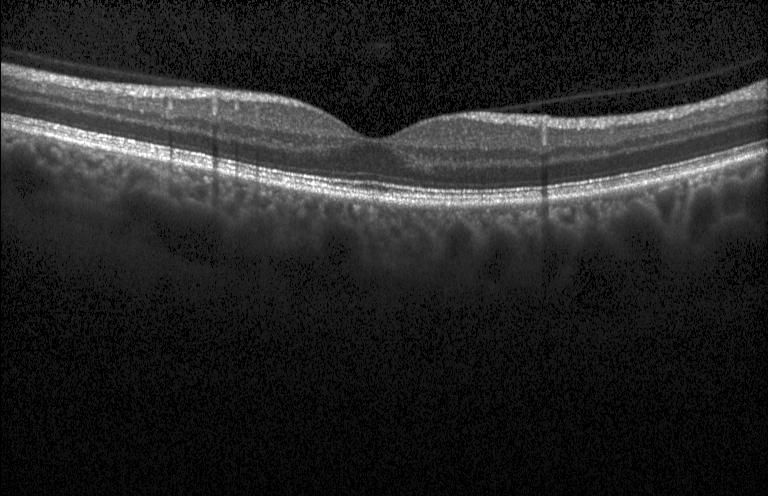 Optical coherence tomography scan · macular scan — Finding: no evidence of CNV, DME, or drusen.